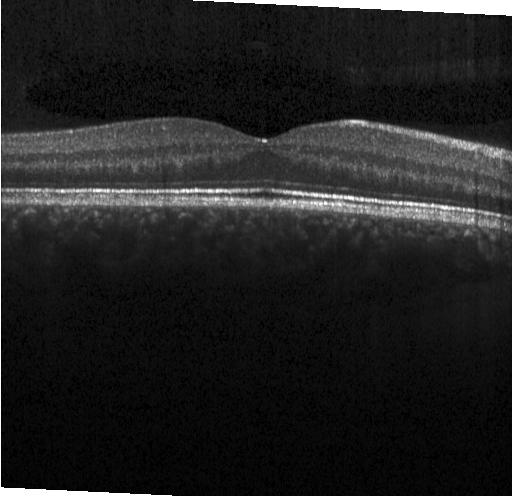

Instrument: Heidelberg Spectralis, retinal OCT cross-section, SD-OCT, through the macula — Finding: neither CNV, DME, nor drusen.